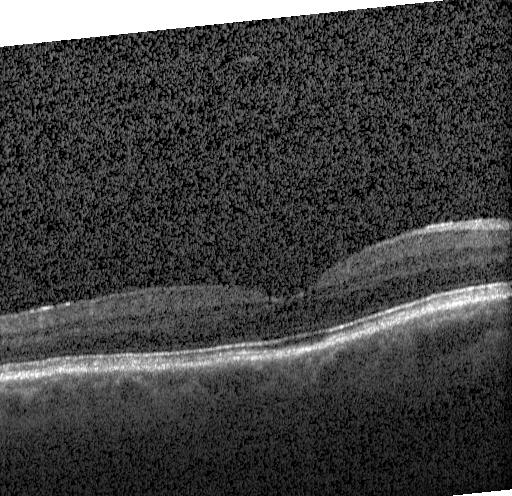
OCT finding: no CNV, no DME, and no drusen.